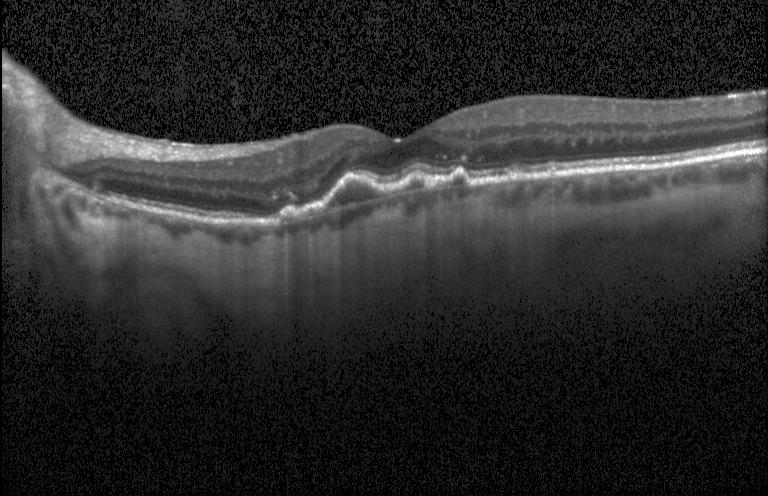
SD-OCT; optical coherence tomography scan — The scan shows choroidal neovascularization (CNV).